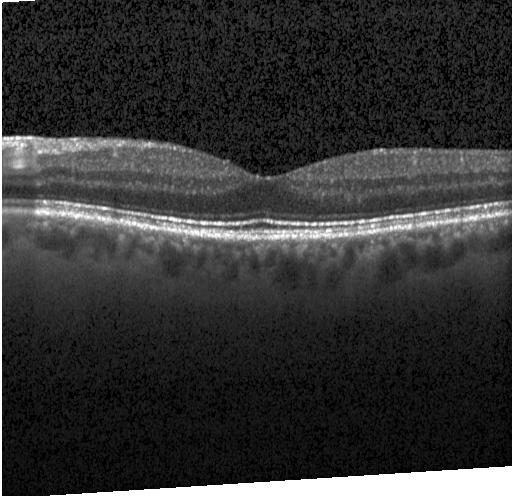
OCT line scan
Assessment: no evidence of choroidal neovascularization, diabetic macular edema, or drusen.